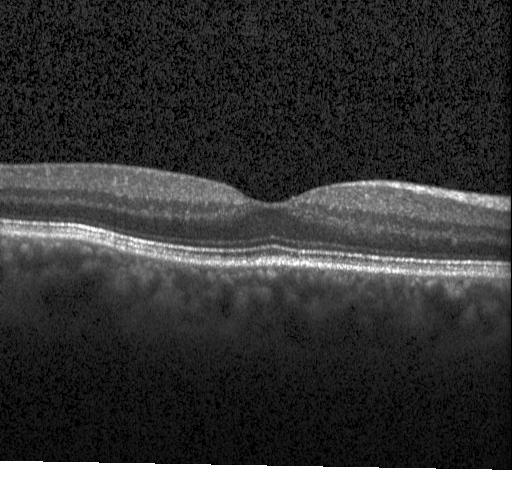 Macular OCT: no evidence of choroidal neovascularization, diabetic macular edema, or drusen.